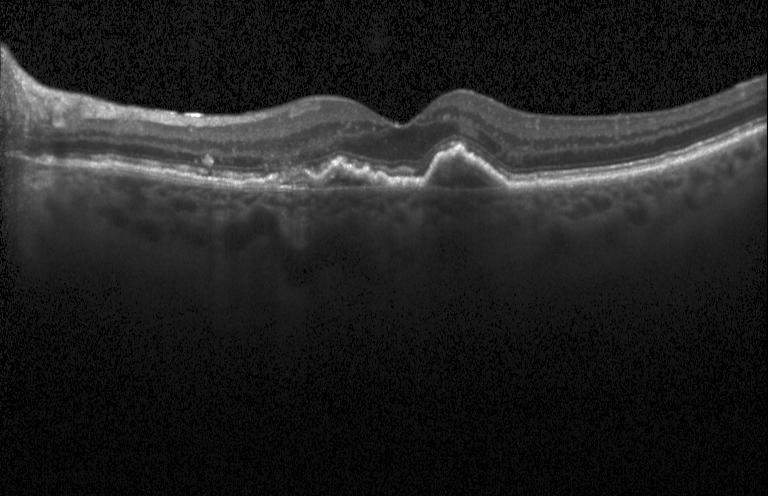
Finding: a choroidal neovascular membrane.